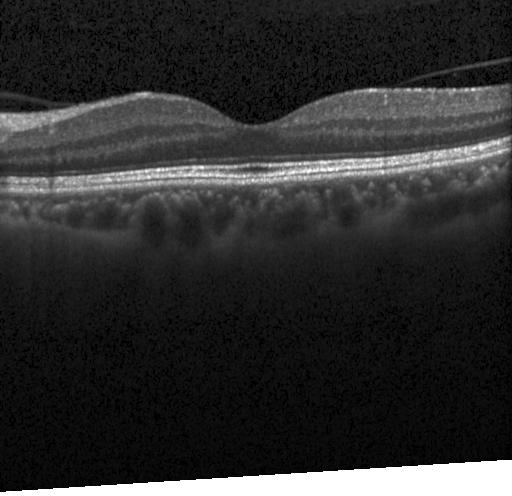
Retinal OCT cross-section.
OCT finding: no choroidal neovascularization, diabetic macular edema, or drusen.